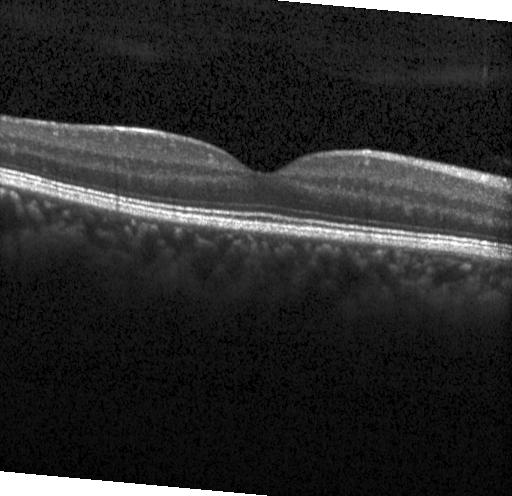

OCT B-scan
No choroidal neovascularization, diabetic macular edema, or drusen.